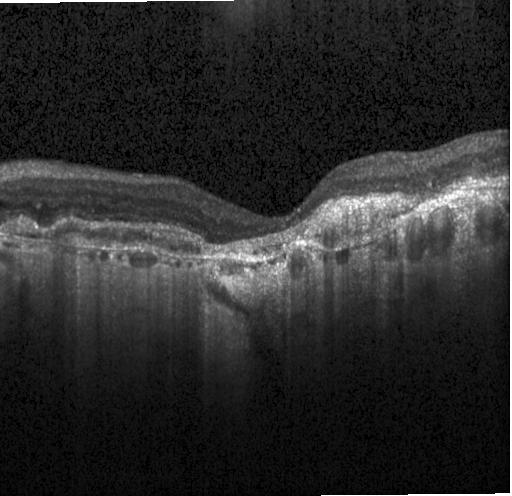 Finding: CNV.